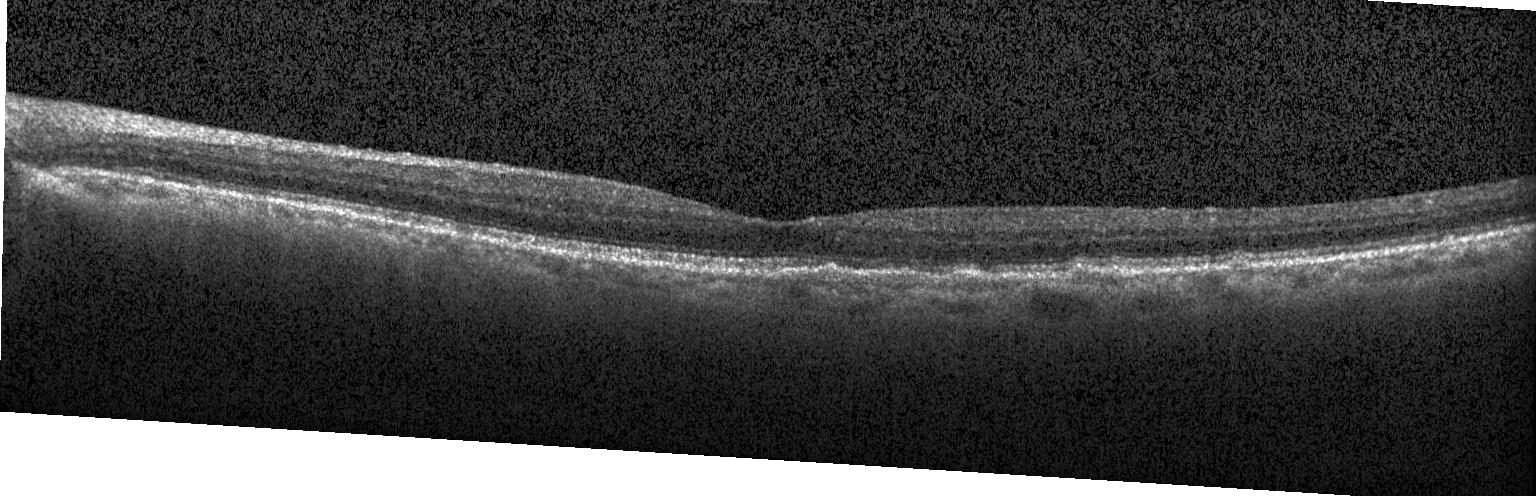

SD-OCT · optical coherence tomography scan · Heidelberg Spectralis OCT system
Multiple drusen.